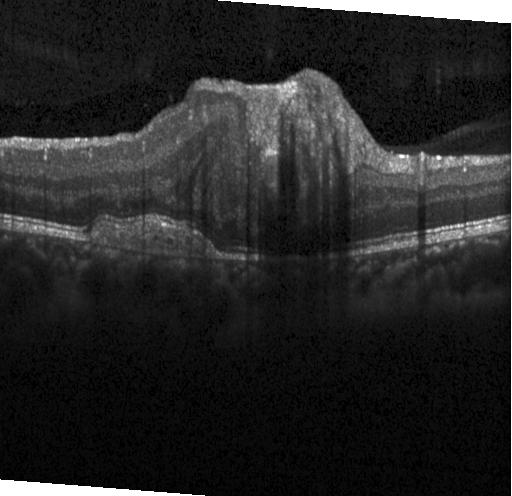 Optical coherence tomography scan
Dx: choroidal neovascularization.